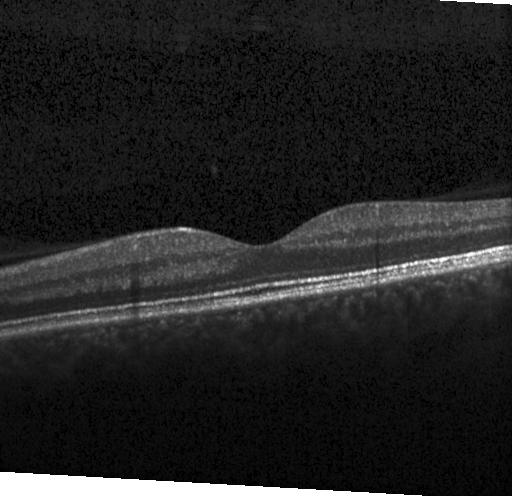

Retinal OCT cross-section
Assessment: neither CNV, DME, nor drusen.